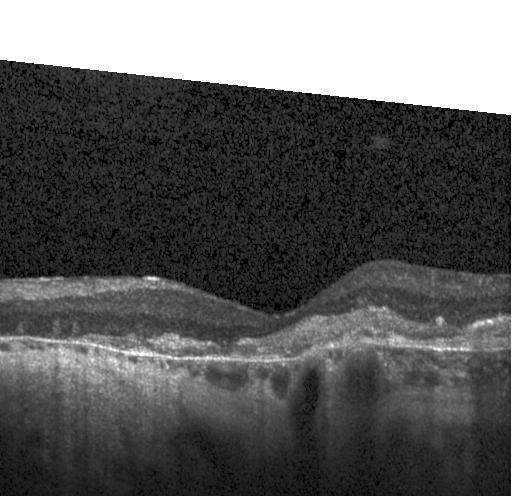
OCT finding: a choroidal neovascular membrane.